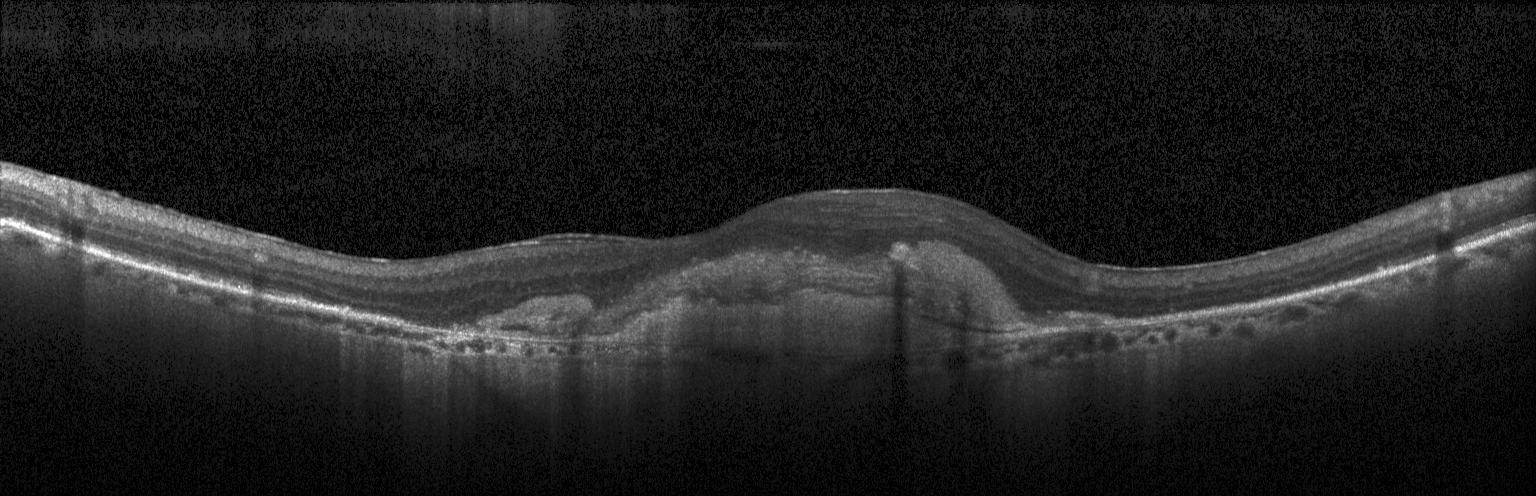
OCT scan showing choroidal neovascularization (CNV).